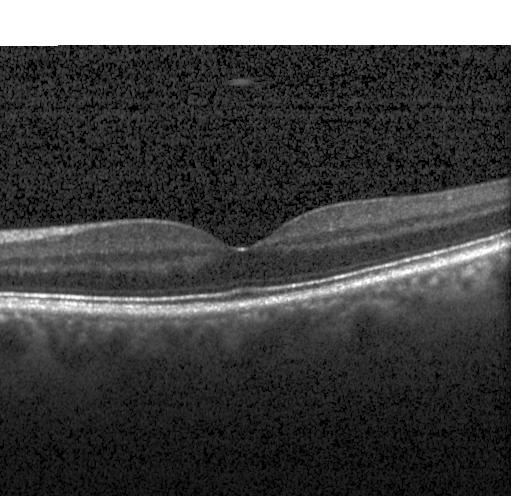

Heidelberg Spectralis · OCT line scan
Diagnosis: no choroidal neovascularization, no diabetic macular edema, and no drusen.